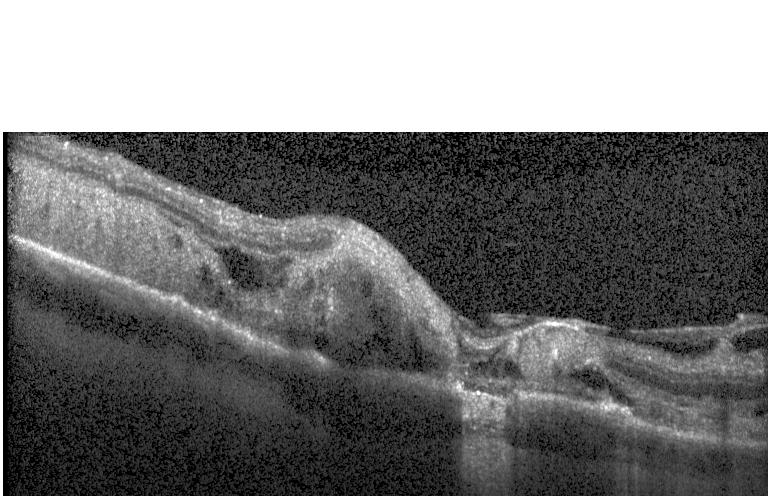

Finding: a choroidal neovascular membrane.